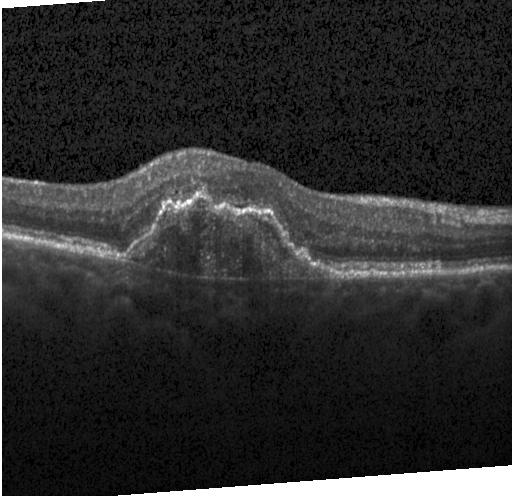
OCT B-scan showing choroidal neovascularization (CNV).